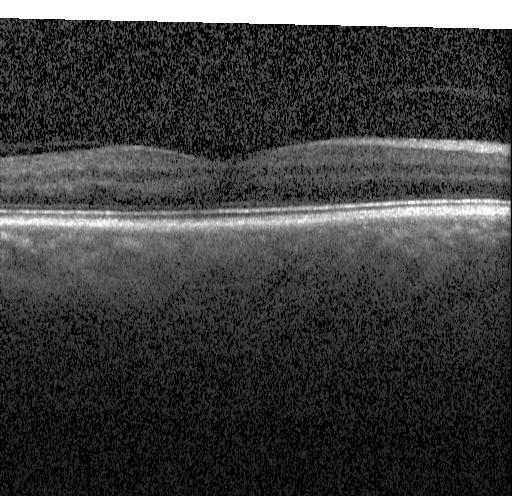 OCT line scan · spectral-domain OCT. Diagnosis: no choroidal neovascularization, diabetic macular edema, or drusen.